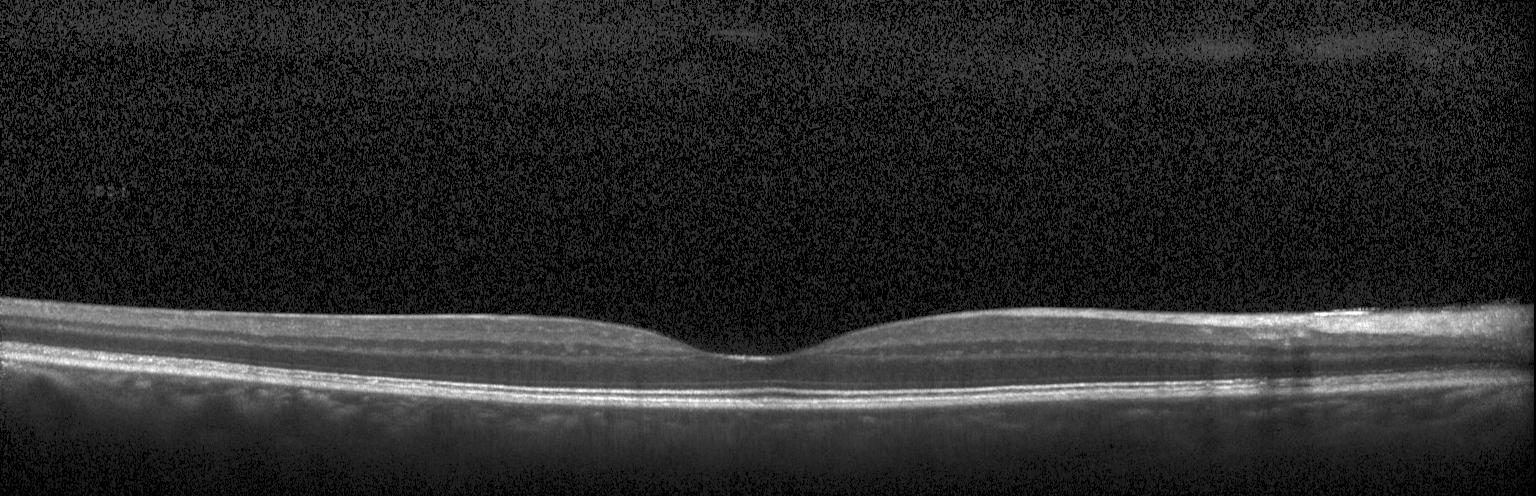

Heidelberg Spectralis · macular scan · spectral-domain OCT · OCT B-scan. Neither choroidal neovascularization, diabetic macular edema, nor drusen.